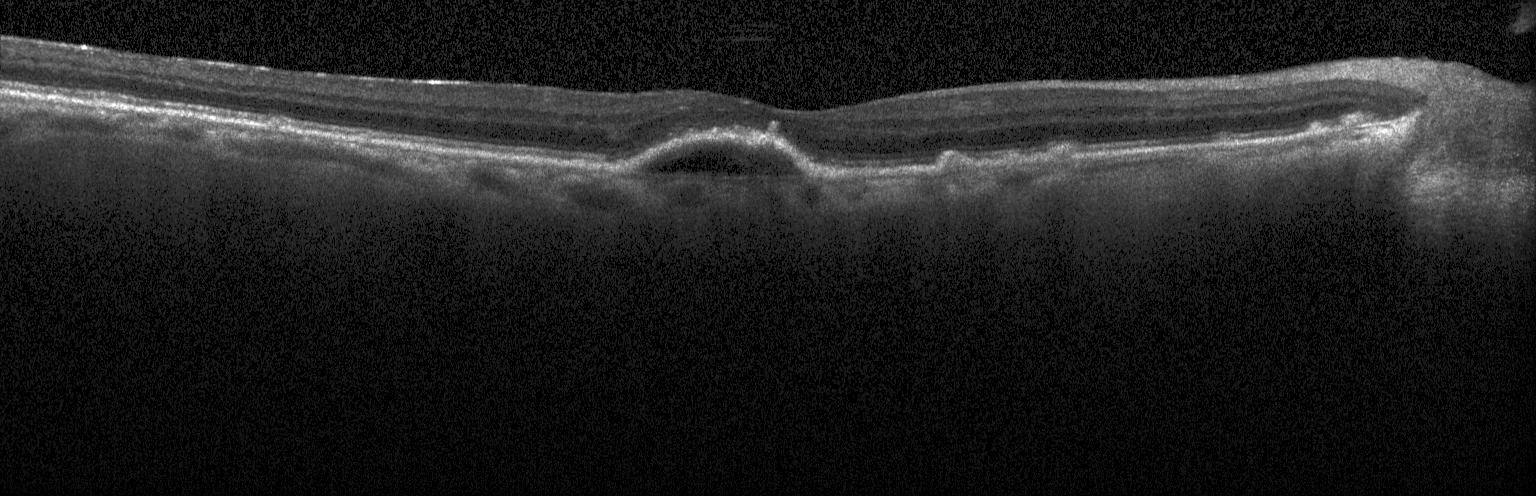
OCT scan showing choroidal neovascularization.